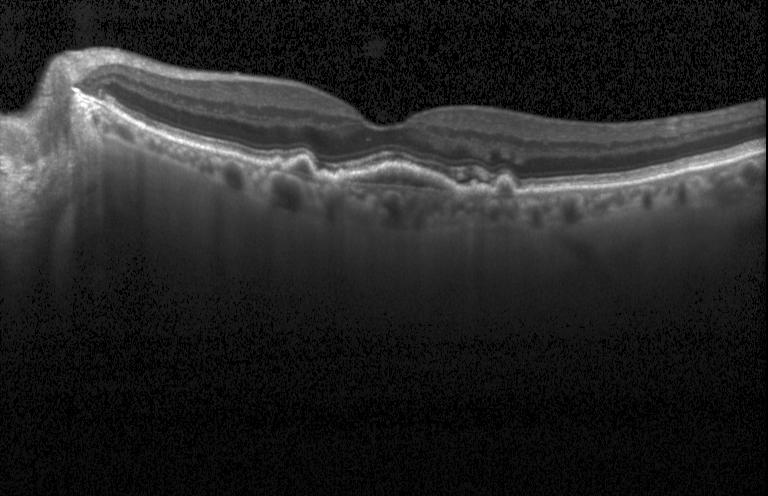

Optical coherence tomography B-scan
The scan shows choroidal neovascularization (CNV).